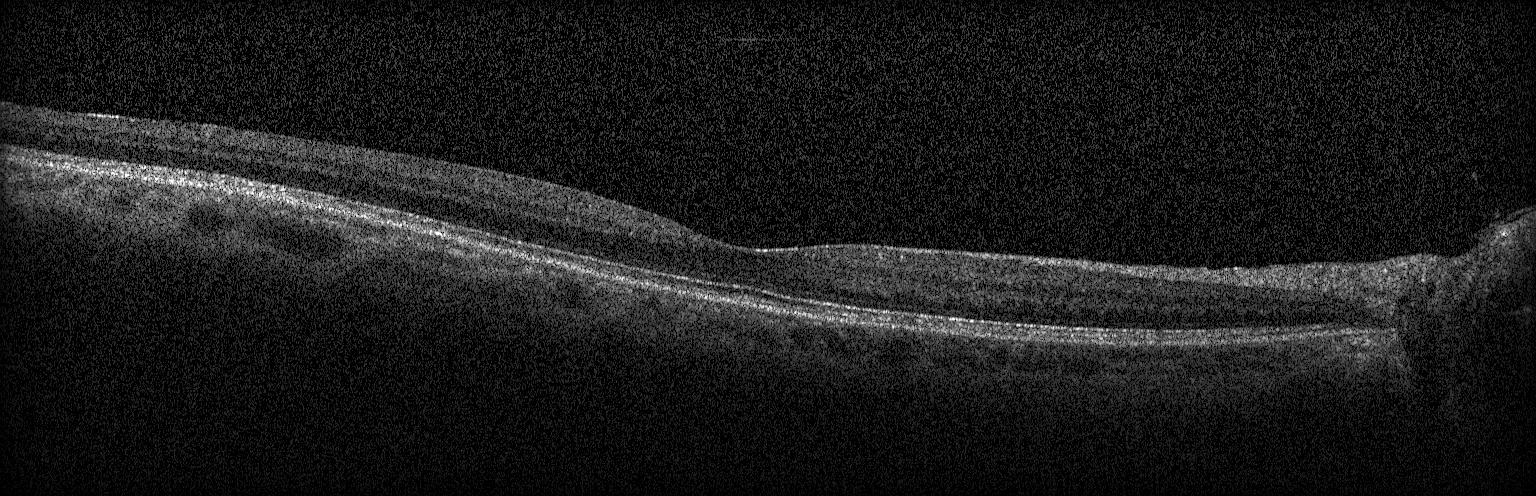

Finding: neither choroidal neovascularization, diabetic macular edema, nor drusen.